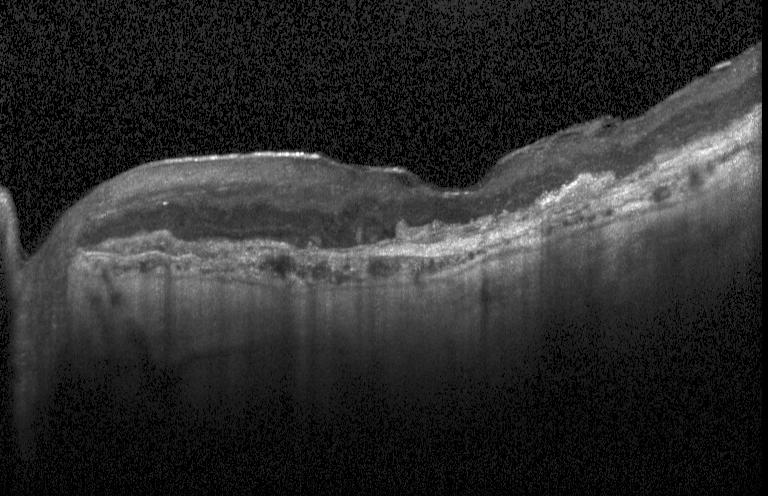 The scan shows CNV.